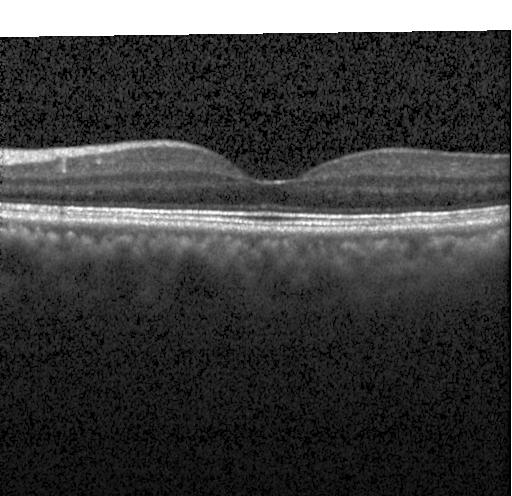 OCT scan showing no choroidal neovascularization, no diabetic macular edema, and no drusen.